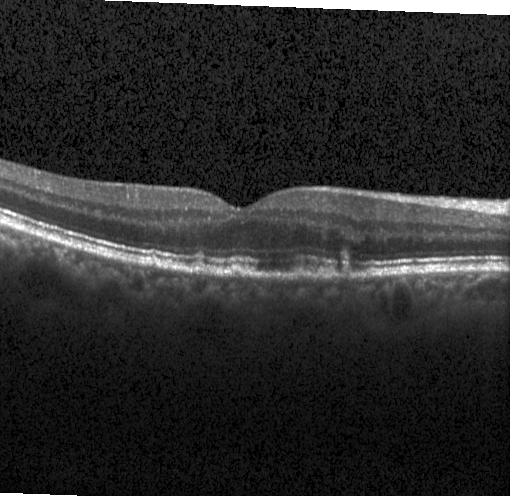 Optical coherence tomography scan; acquired on a Heidelberg Spectralis.
Diagnosis: multiple drusen.